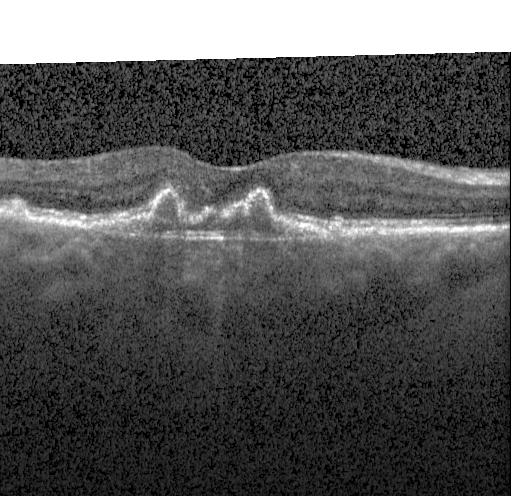
Optical coherence tomography scan. Finding: choroidal neovascularization.